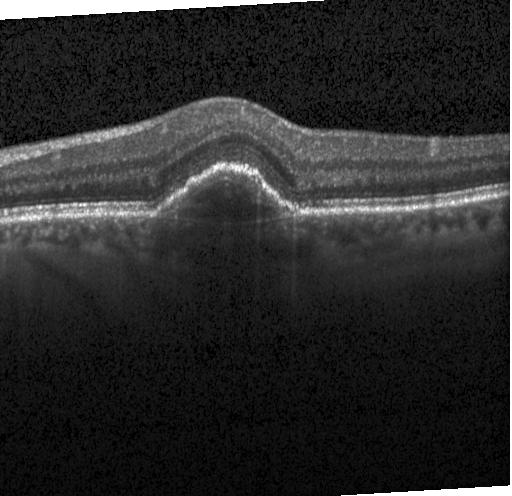 Assessment: a choroidal neovascular membrane.